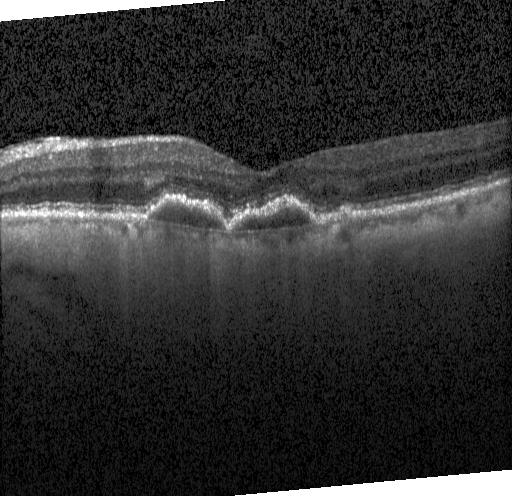

Acquired on a Heidelberg Spectralis; horizontal scan through the fovea; OCT line scan; spectral-domain OCT.
Diagnosis: a choroidal neovascular membrane.